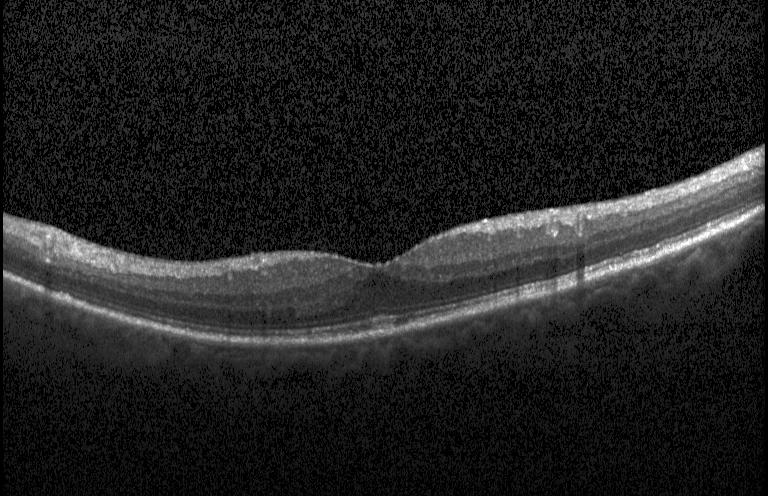 Optical coherence tomography B-scan; SD-OCT; horizontal scan through the fovea; instrument: Heidelberg Spectralis.
Macular OCT: no evidence of choroidal neovascularization, diabetic macular edema, or drusen.